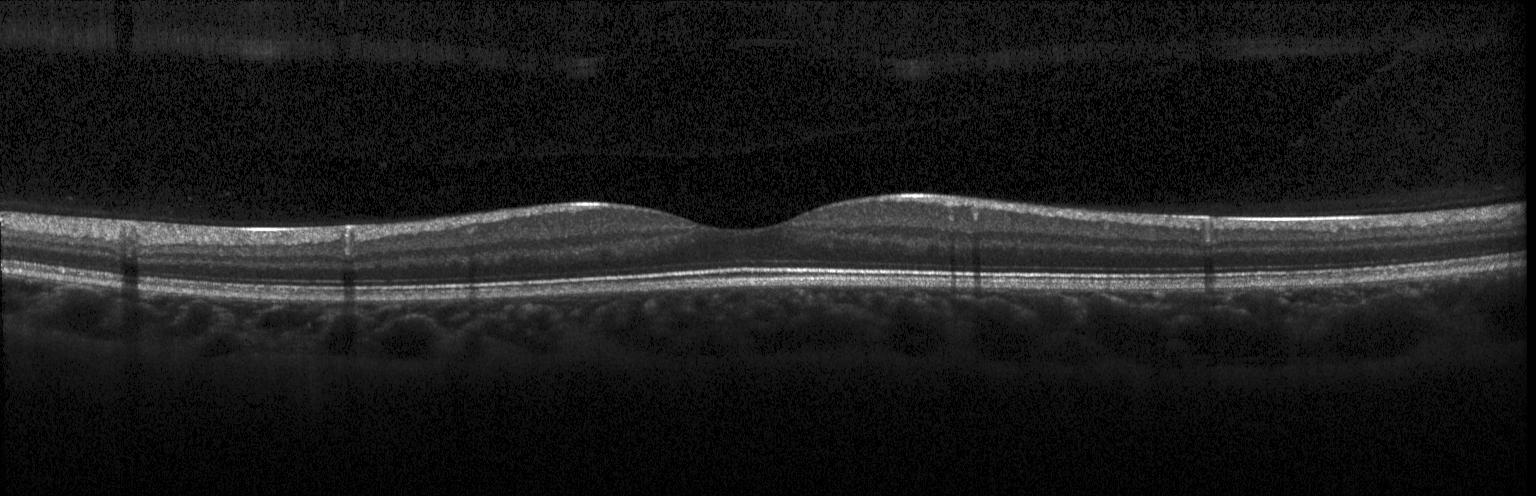 Diagnosis: no choroidal neovascularization, diabetic macular edema, or drusen.